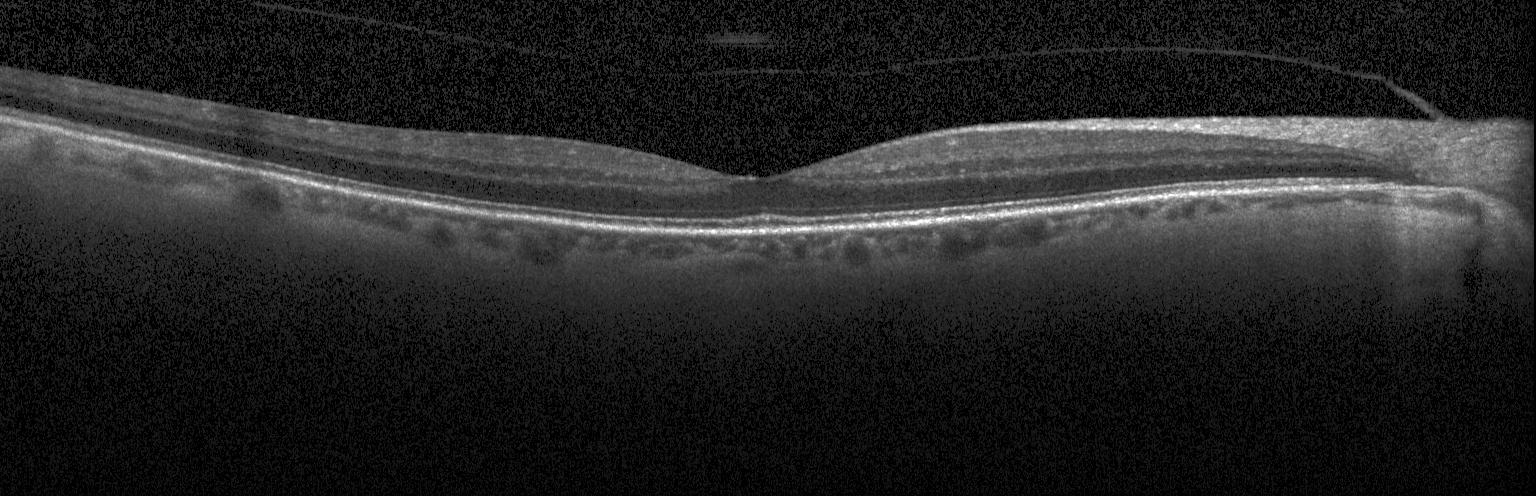

Spectral-domain OCT. Retinal OCT cross-section — Impression: no CNV, no DME, and no drusen.